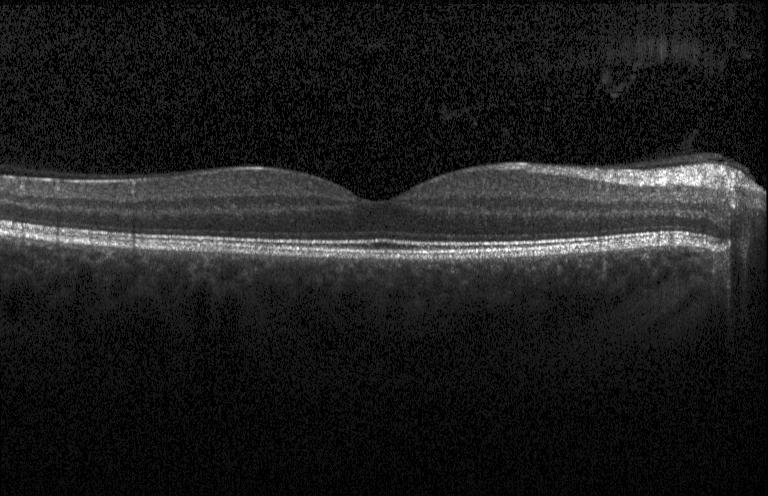

Impression: no choroidal neovascularization, no diabetic macular edema, and no drusen.